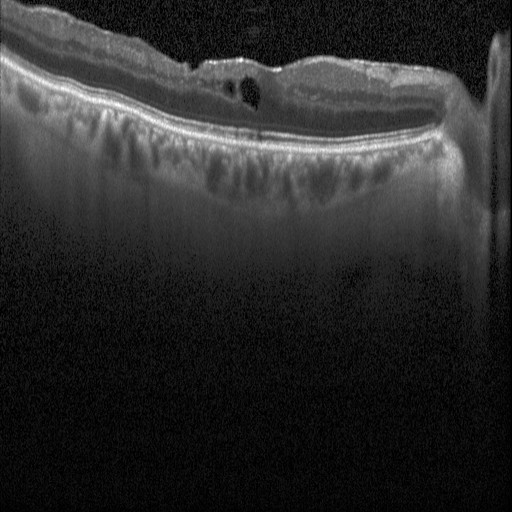 Assessment: diabetic macular edema.